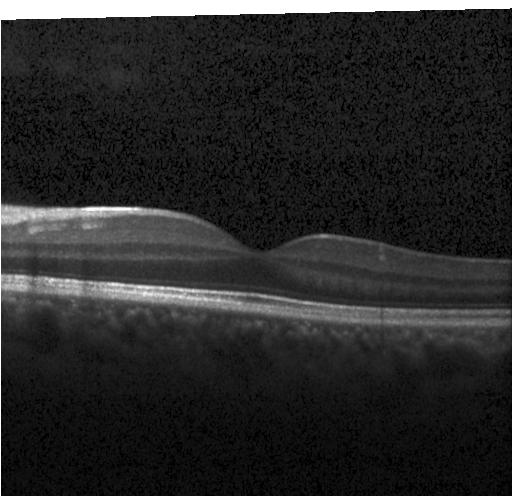

Optical coherence tomography scan.
Finding: no choroidal neovascularization, diabetic macular edema, or drusen.